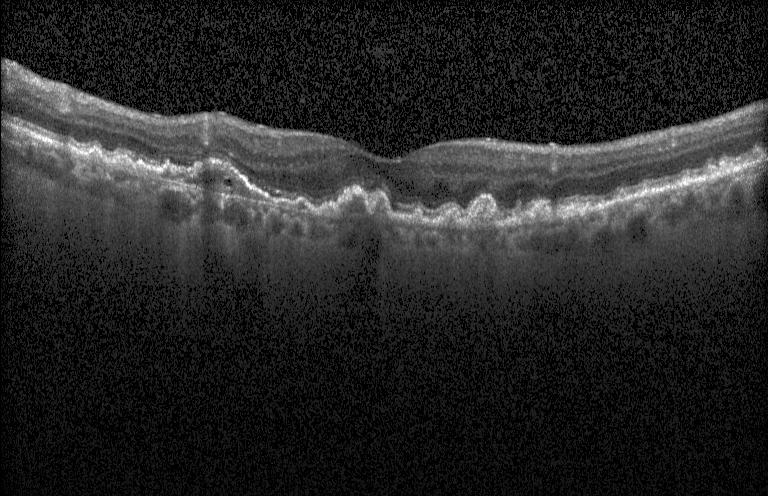 OCT B-scan; fovea-centered. Drusen.